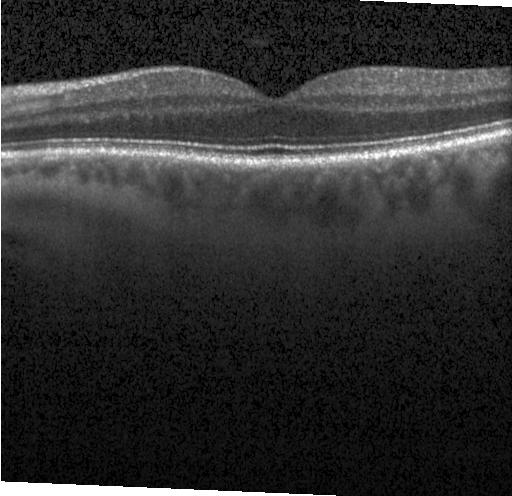 Assessment: no choroidal neovascularization, no diabetic macular edema, and no drusen.